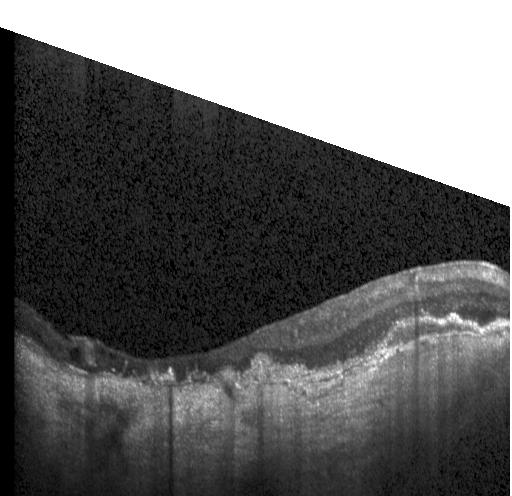 Impression: a choroidal neovascular membrane.